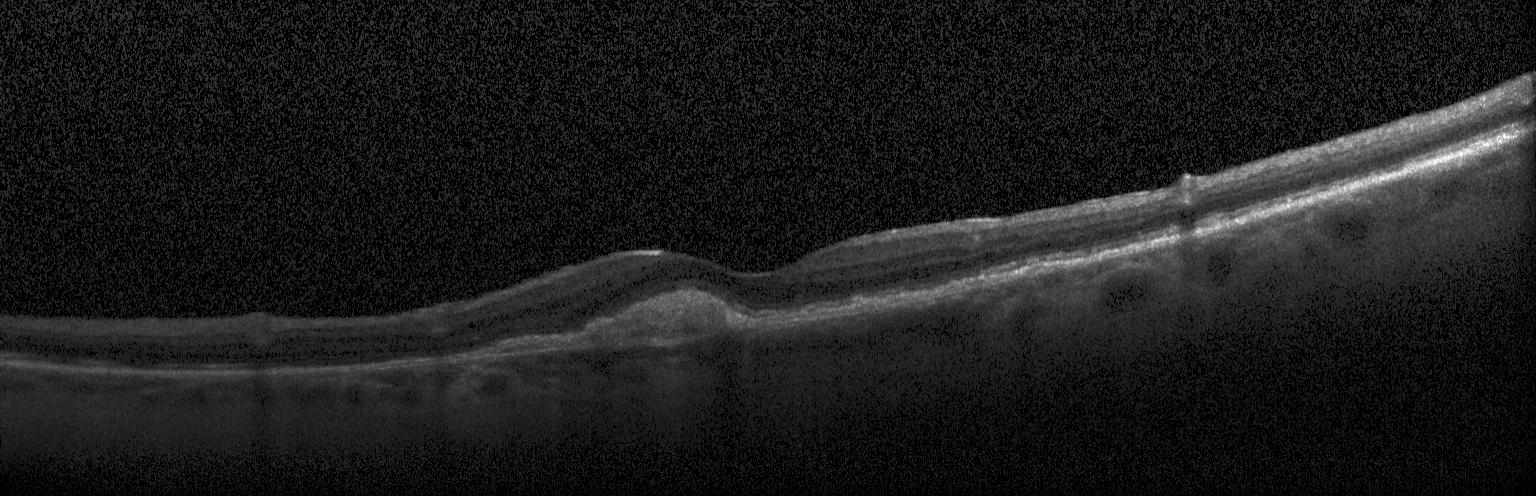

Optical coherence tomography B-scan
Macular OCT: a choroidal neovascular membrane.